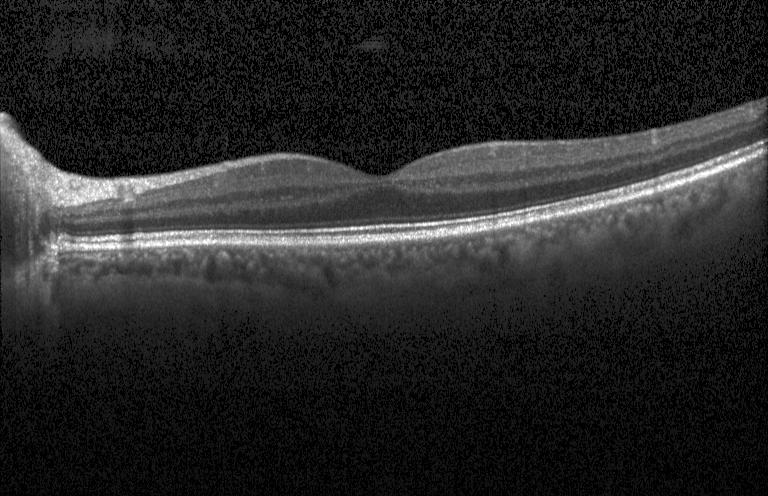

OCT B-scan showing no CNV, no DME, and no drusen.